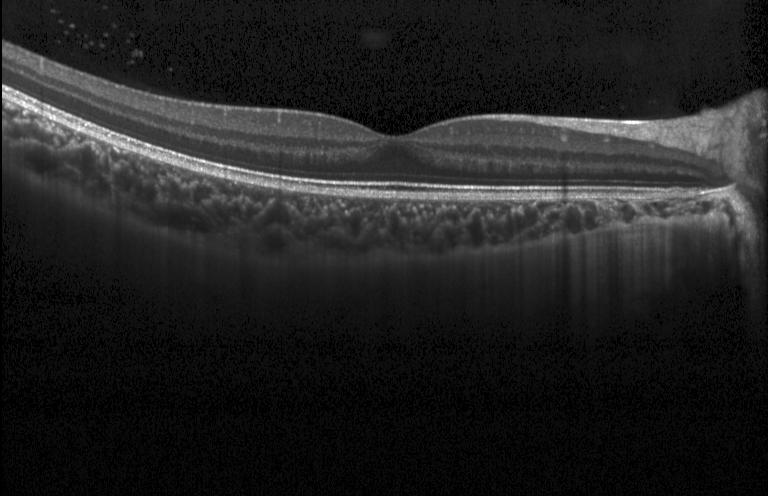
Diagnosis: no CNV, no DME, and no drusen.